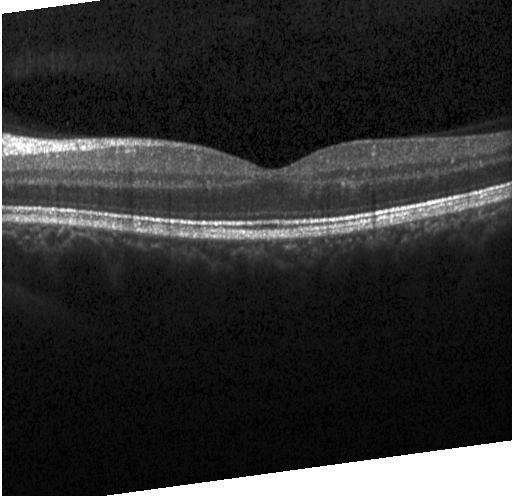

Optical coherence tomography B-scan.
Neither choroidal neovascularization, diabetic macular edema, nor drusen.